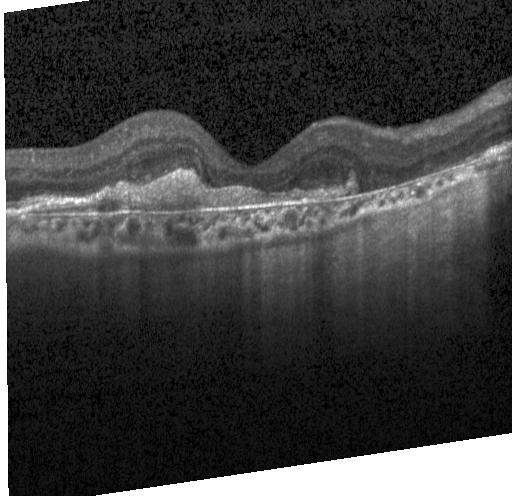

Acquired on a Heidelberg Spectralis, retinal OCT B-scan, fovea-centered, spectral-domain OCT
Assessment: choroidal neovascularization.